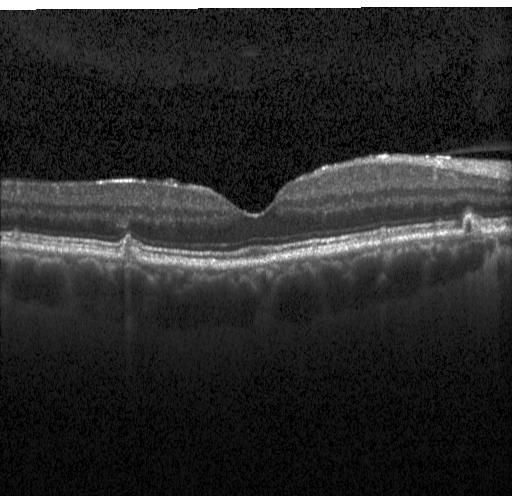
Centered on the fovea; optical coherence tomography B-scan — OCT finding: multiple drusen.